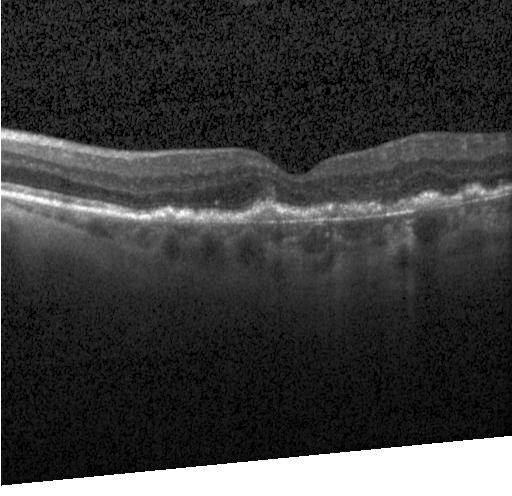 Optical coherence tomography B-scan. Heidelberg Spectralis.
OCT finding: a choroidal neovascular membrane.